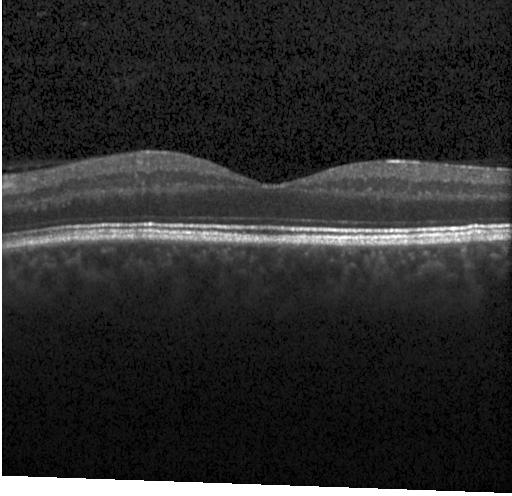 Horizontal scan through the fovea; retinal OCT cross-section — The scan shows neither CNV, DME, nor drusen.